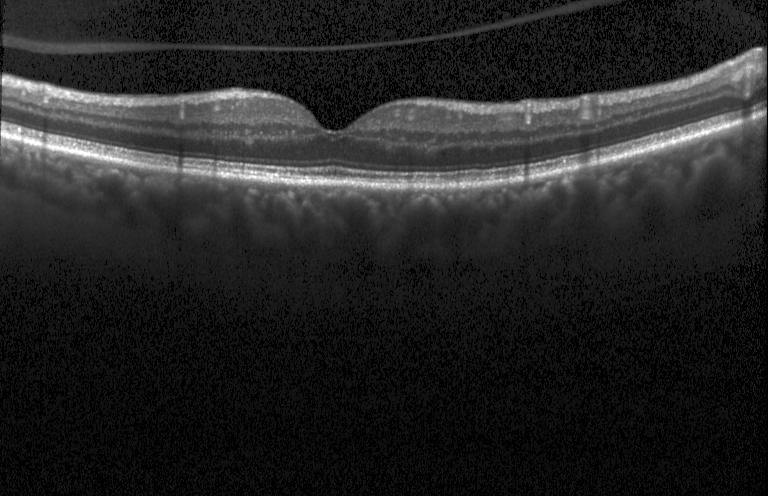

Spectral-domain OCT B-scan: no evidence of choroidal neovascularization, diabetic macular edema, or drusen.